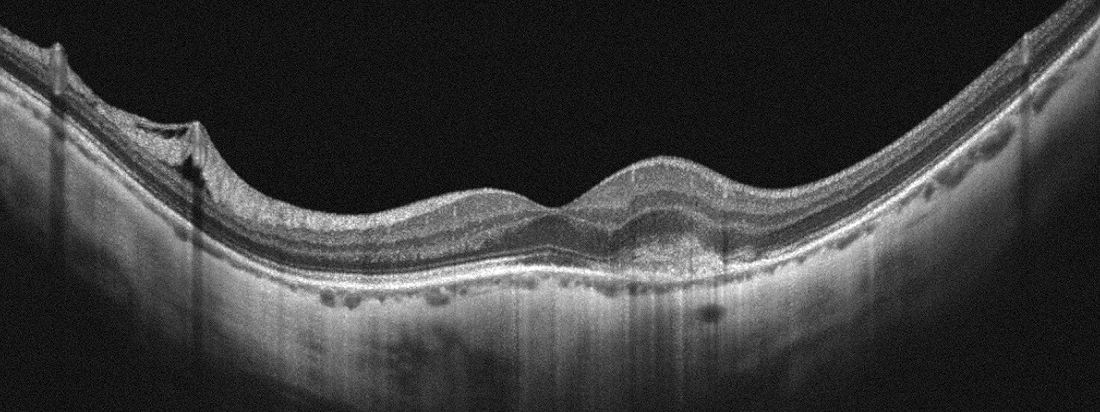 Macular OCT demonstrating age-related macular degeneration.